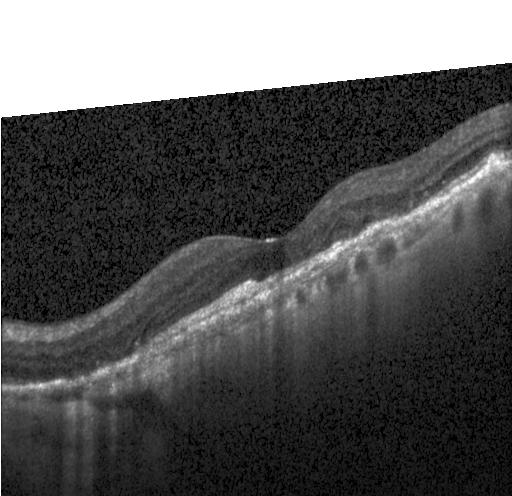

Spectral-domain optical coherence tomography. Through the macula. OCT B-scan. Choroidal neovascularization.